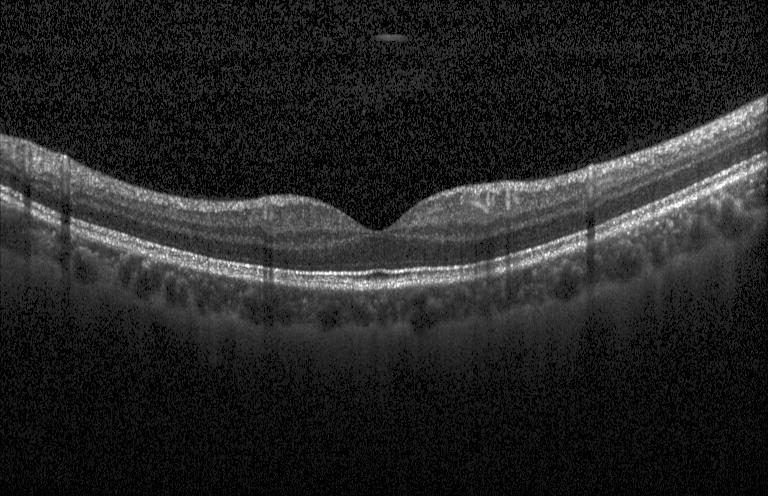
OCT scan showing neither CNV, DME, nor drusen.